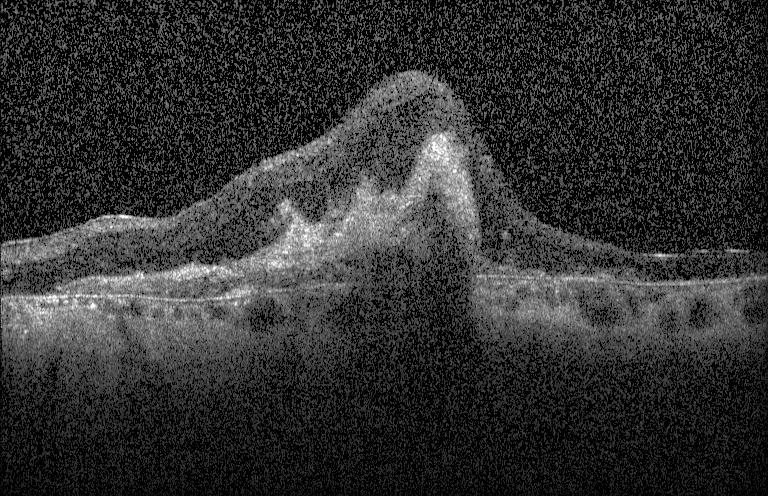
A choroidal neovascular membrane.